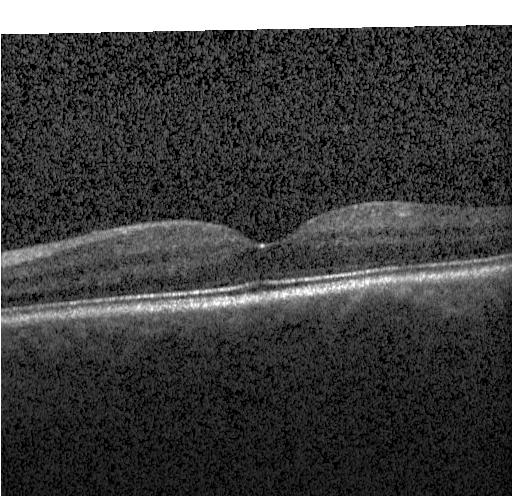 Heidelberg Spectralis OCT system · spectral-domain optical coherence tomography · optical coherence tomography scan — This B-scan demonstrates no CNV, DME, or drusen.